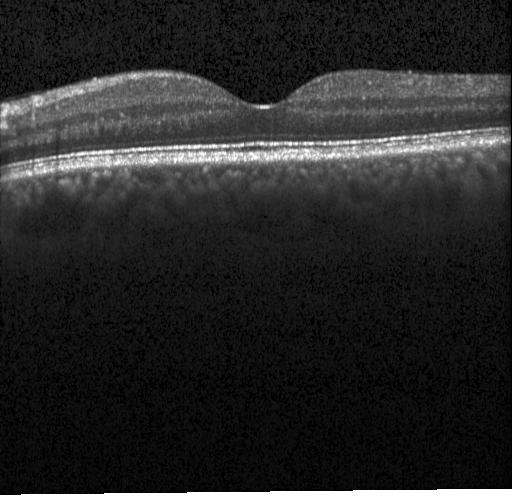
Optical coherence tomography B-scan · through the macula. Finding: no choroidal neovascularization, diabetic macular edema, or drusen.